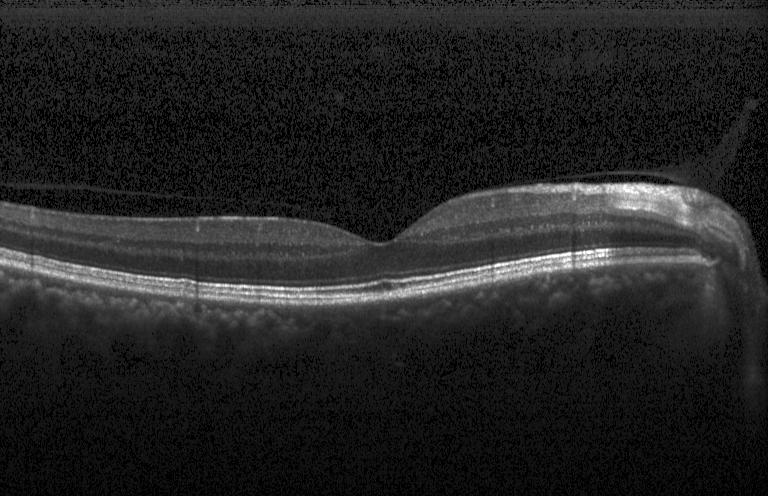

OCT B-scan
Diagnosis: no choroidal neovascularization, diabetic macular edema, or drusen.